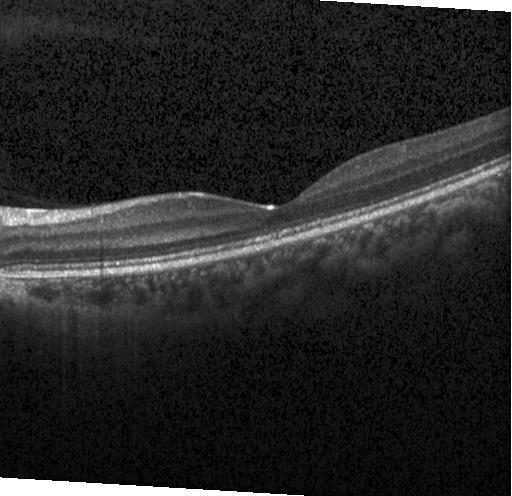
OCT scan showing no evidence of choroidal neovascularization, diabetic macular edema, or drusen.